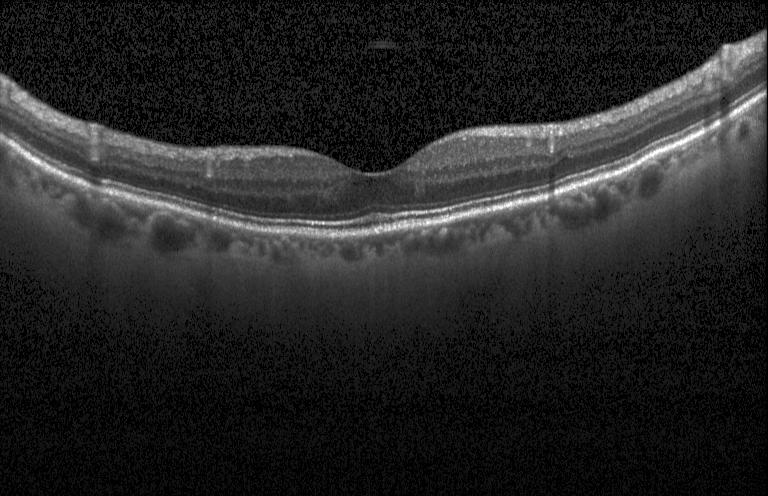 Finding: neither choroidal neovascularization, diabetic macular edema, nor drusen.